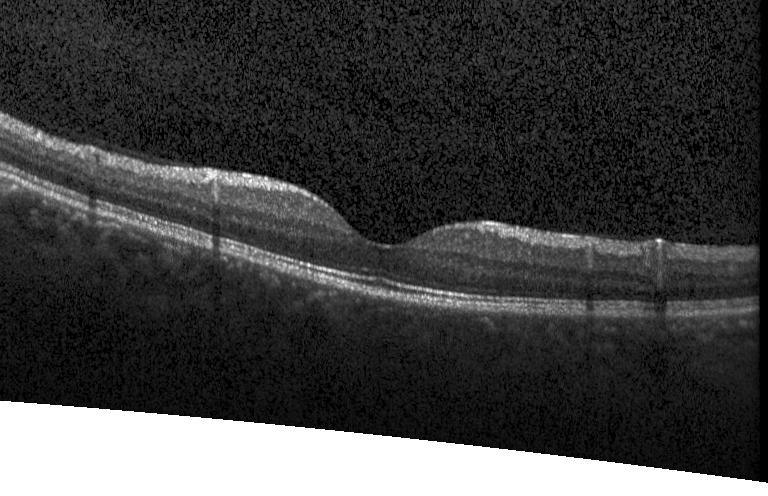
OCT B-scan showing no evidence of choroidal neovascularization, diabetic macular edema, or drusen.